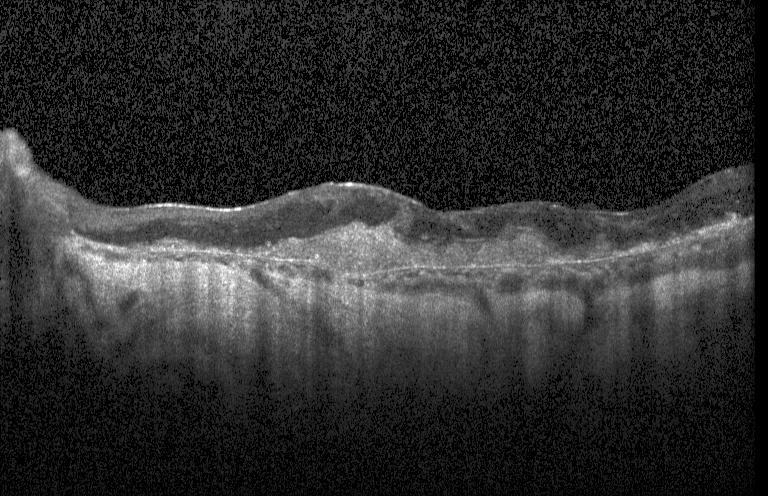 SD-OCT, retinal OCT B-scan, centered on the fovea
The scan shows a choroidal neovascular membrane.